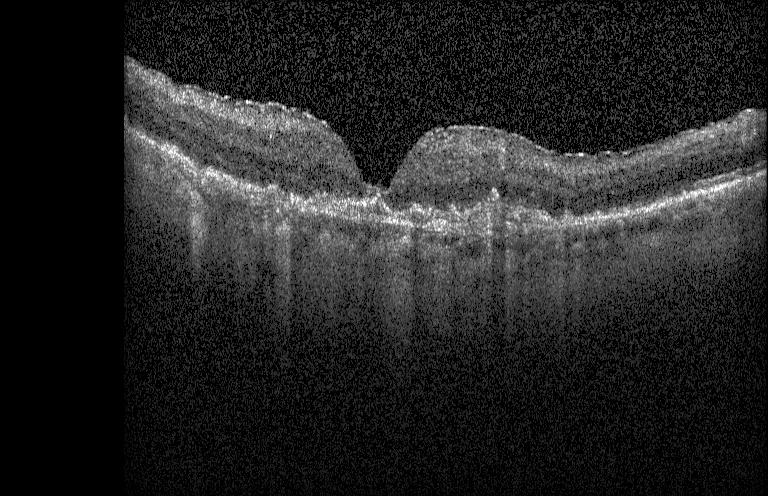 Impression: CNV.